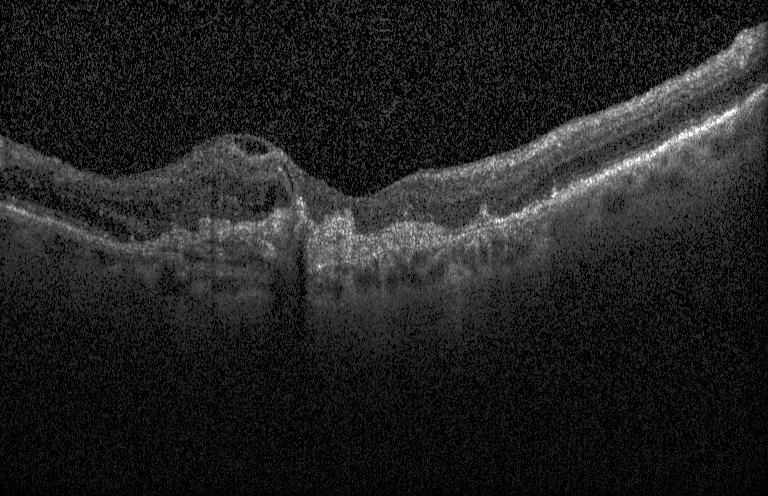
Instrument: Heidelberg Spectralis · optical coherence tomography B-scan. Finding: a choroidal neovascular membrane.